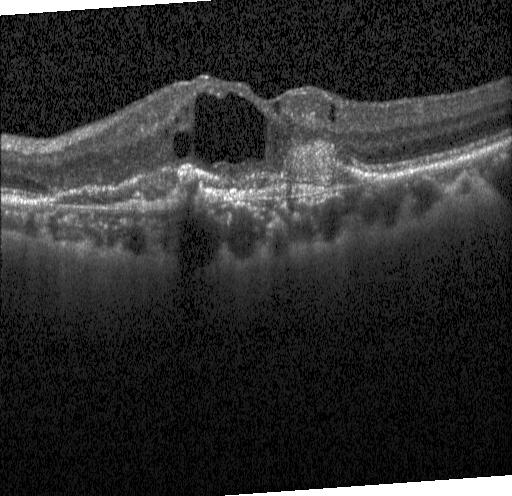
Diagnosis: a choroidal neovascular membrane.